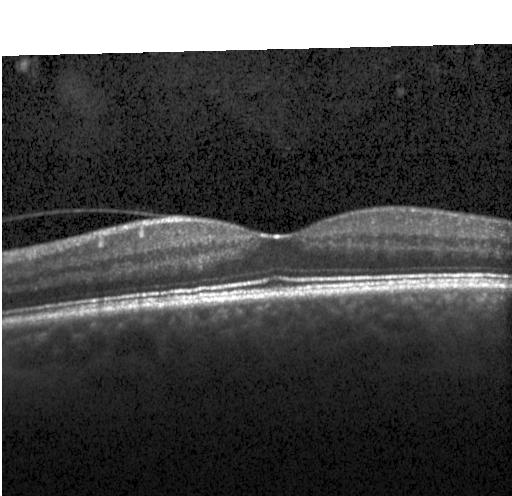 Fovea-centered · SD-OCT · optical coherence tomography scan
This B-scan demonstrates no choroidal neovascularization, no diabetic macular edema, and no drusen.